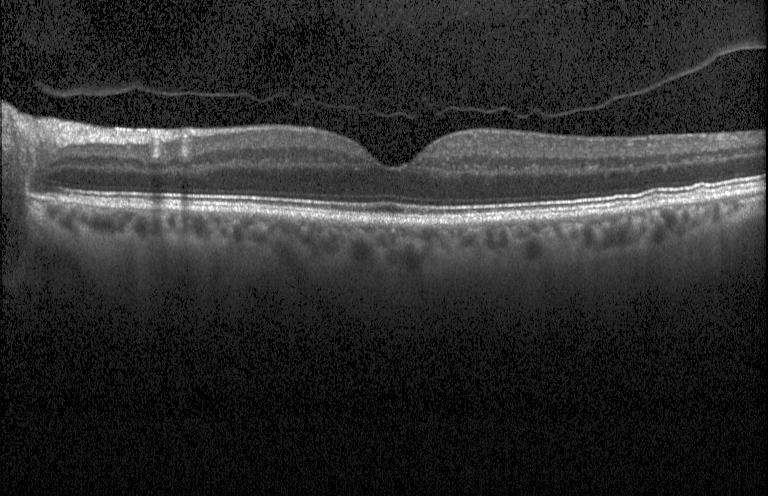 OCT scan showing no choroidal neovascularization, diabetic macular edema, or drusen.